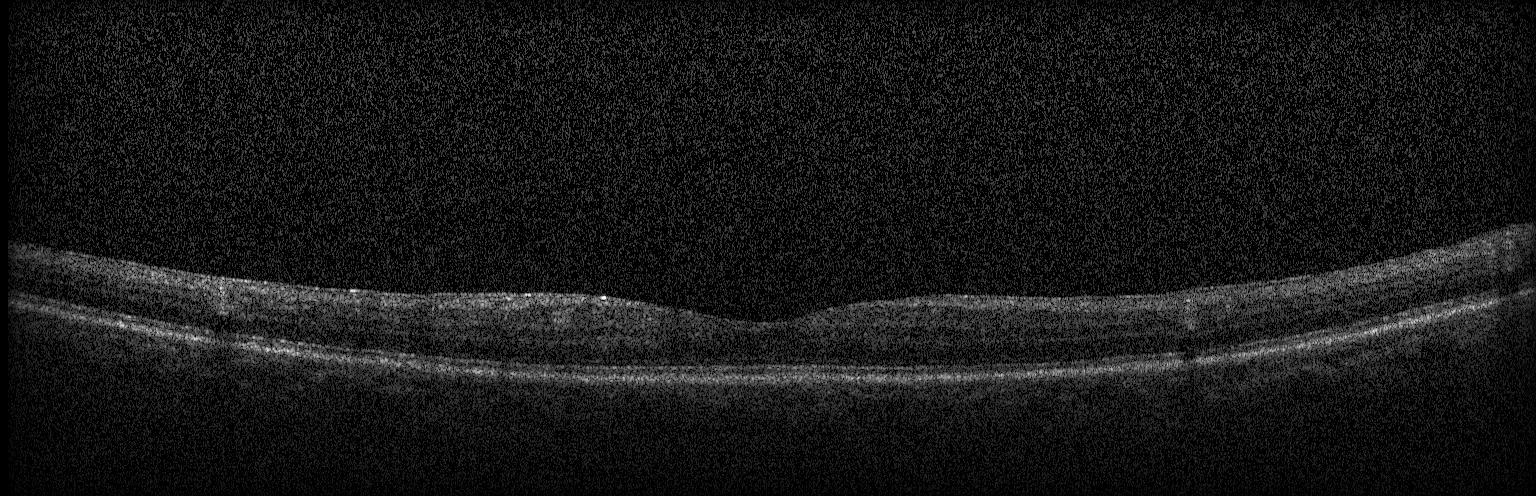

OCT line scan. Acquired on a Heidelberg Spectralis. Macular scan. Spectral-domain OCT — Diagnosis: neither choroidal neovascularization, diabetic macular edema, nor drusen.